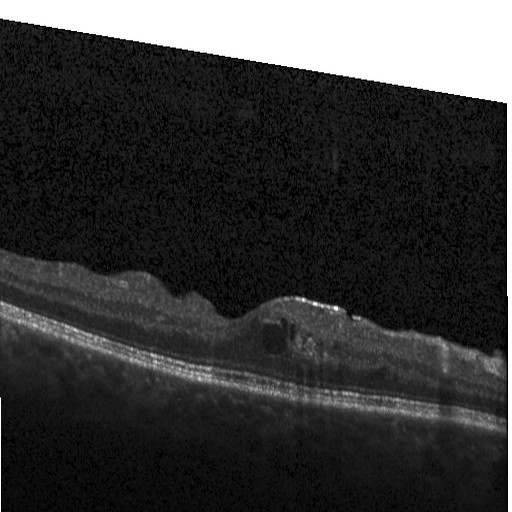
Spectral-domain optical coherence tomography, through the macula, retinal OCT cross-section, Heidelberg Spectralis.
Finding: DME.